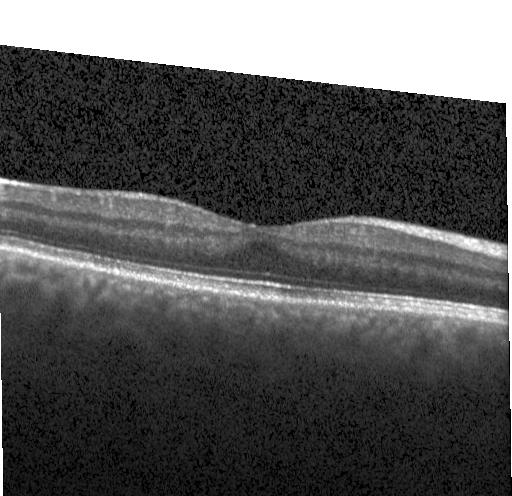 OCT finding: neither CNV, DME, nor drusen.